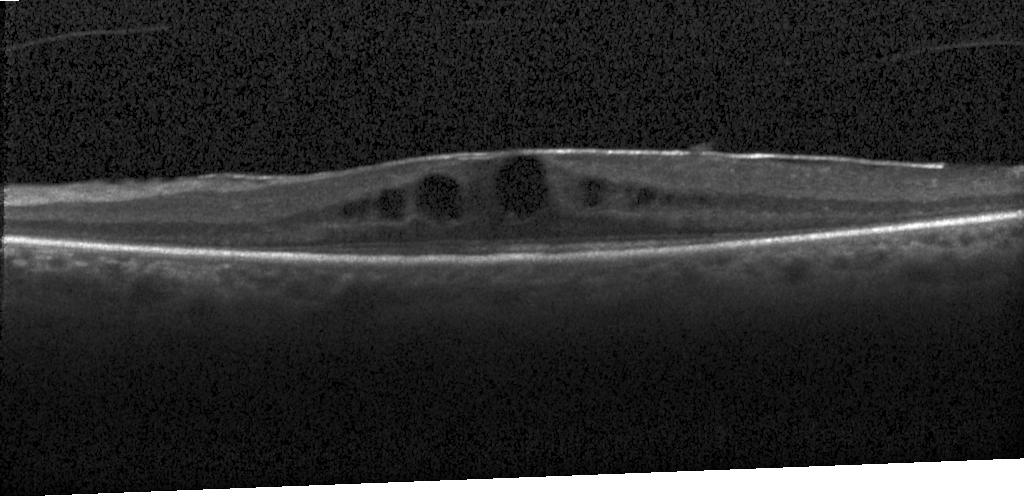 OCT B-scan.
Dx: DME.